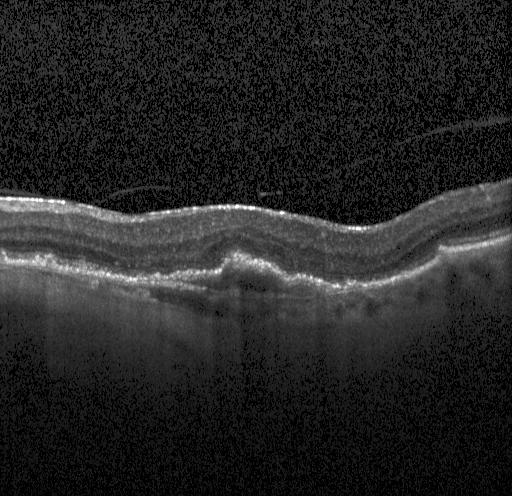

Finding: choroidal neovascularization (CNV).